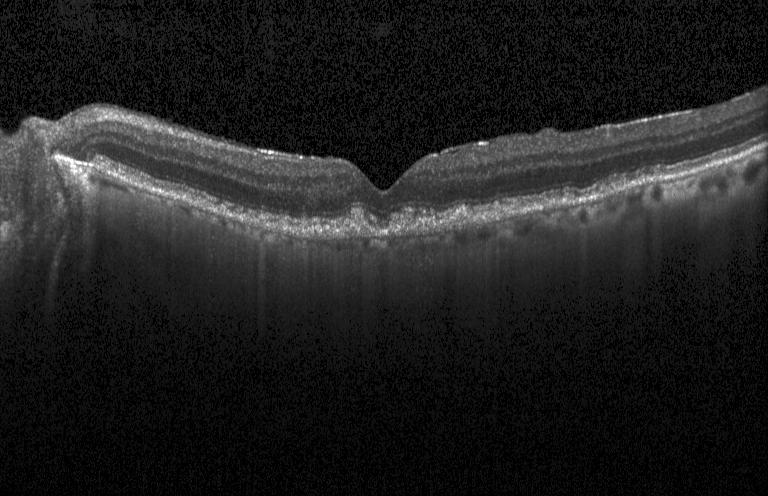

Diagnosis: sub-RPE drusenoid deposits.